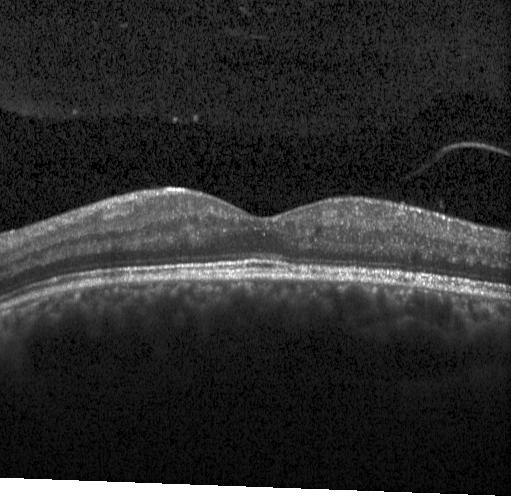 OCT finding: no CNV, DME, or drusen.